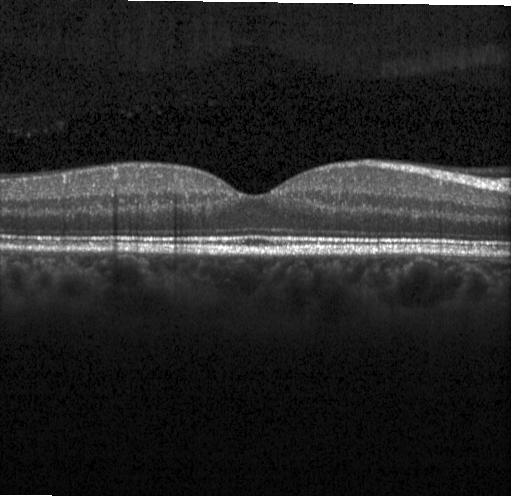 Instrument: Heidelberg Spectralis · SD-OCT · retinal OCT B-scan
Diagnosis: no choroidal neovascularization, diabetic macular edema, or drusen.